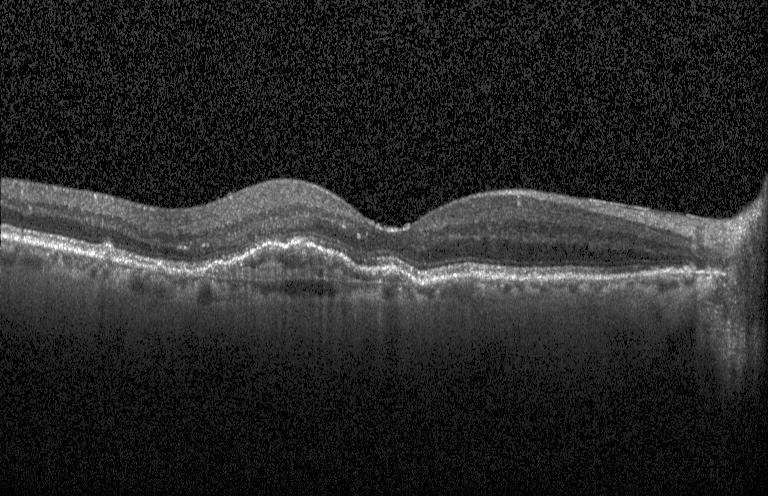 Retinal OCT cross-section.
Impression: choroidal neovascularization (CNV).